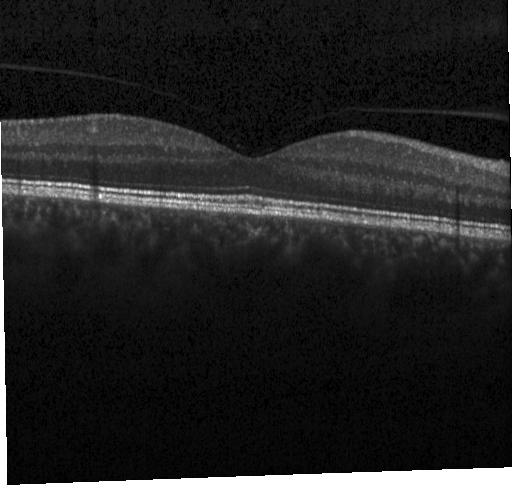
OCT scan showing neither choroidal neovascularization, diabetic macular edema, nor drusen.